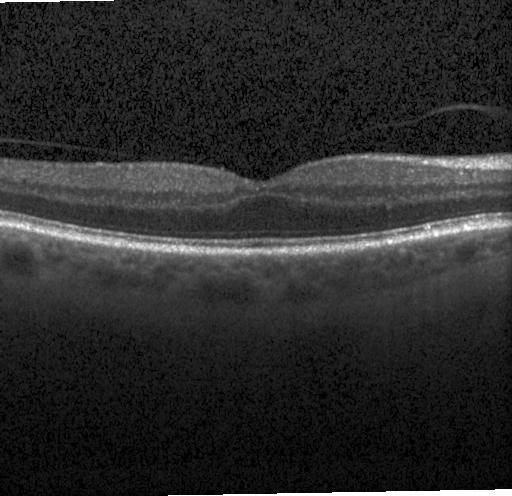
No CNV, DME, or drusen.